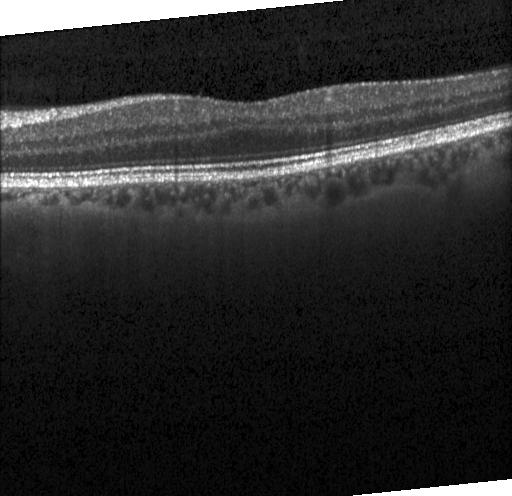 Retinal OCT cross-section showing no CNV, DME, or drusen.